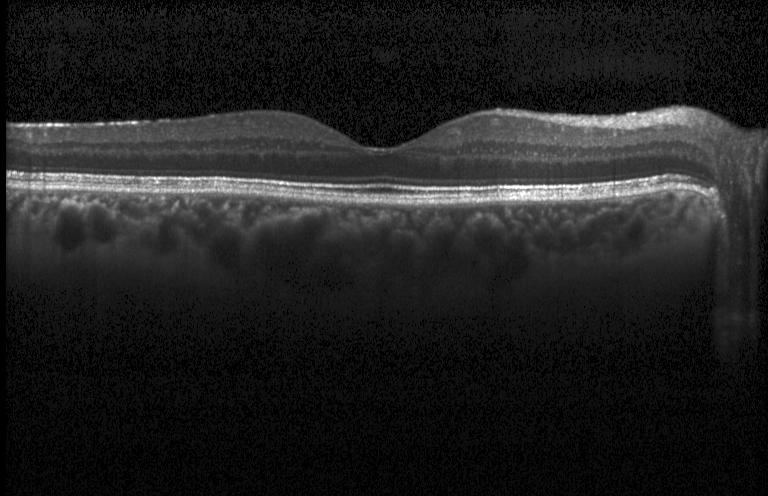
Dx: no choroidal neovascularization, diabetic macular edema, or drusen.